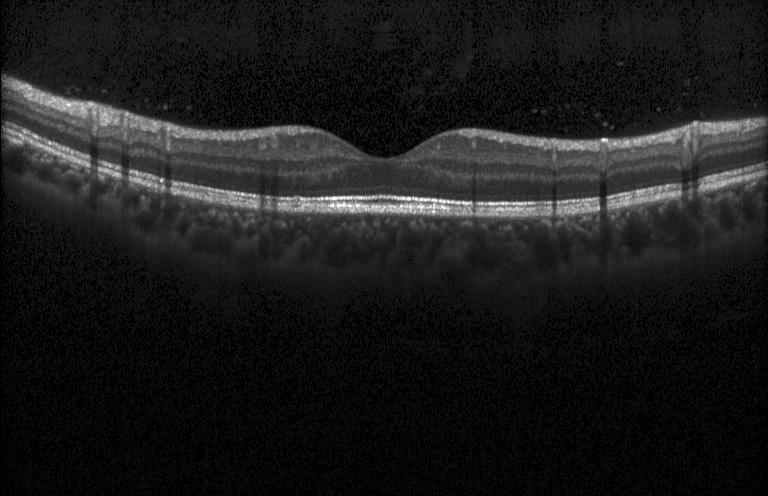 Optical coherence tomography B-scan · spectral-domain optical coherence tomography · fovea-centered.
Macular OCT: neither choroidal neovascularization, diabetic macular edema, nor drusen.